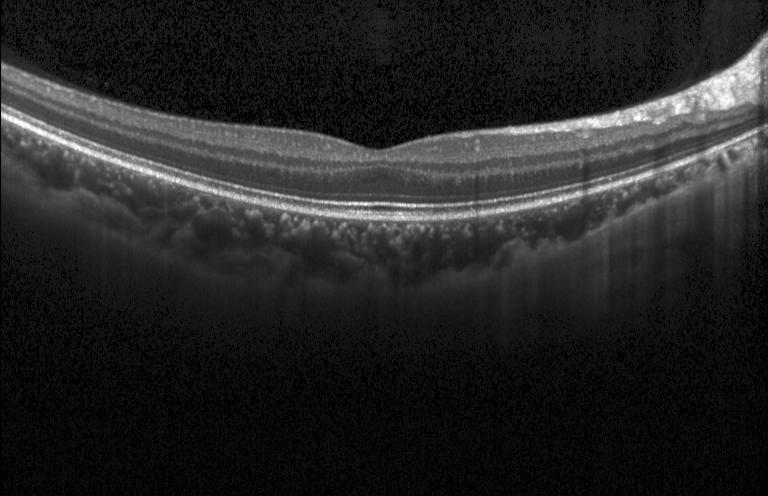 Diagnosis: no choroidal neovascularization, diabetic macular edema, or drusen.